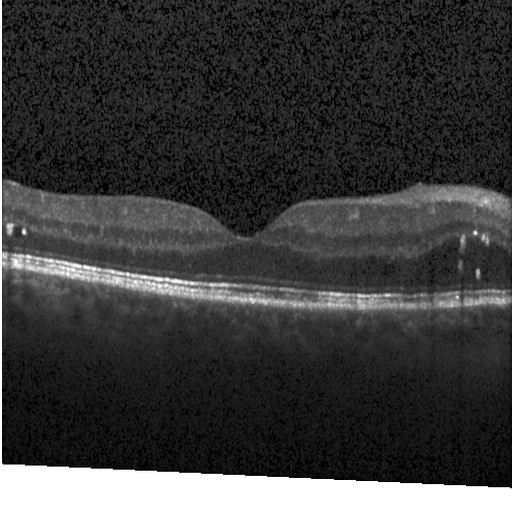 Retinal OCT B-scan — Finding: diabetic macular edema (DME).